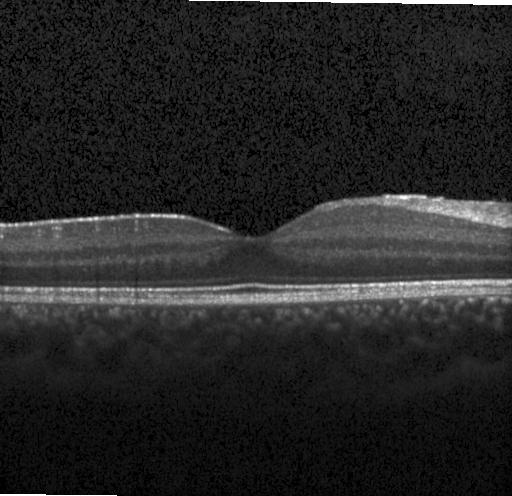
Acquired on a Heidelberg Spectralis · optical coherence tomography scan · through the macula
OCT finding: no evidence of CNV, DME, or drusen.